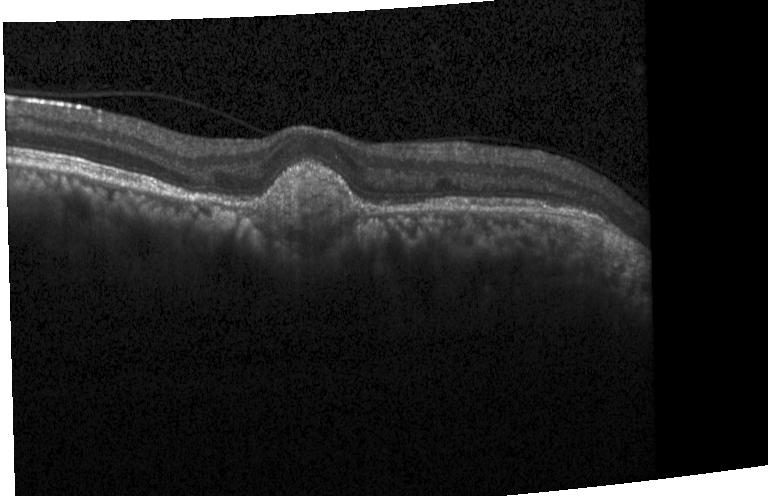

Acquired on a Heidelberg Spectralis · macular scan · optical coherence tomography B-scan · spectral-domain optical coherence tomography.
Dx: a choroidal neovascular membrane.